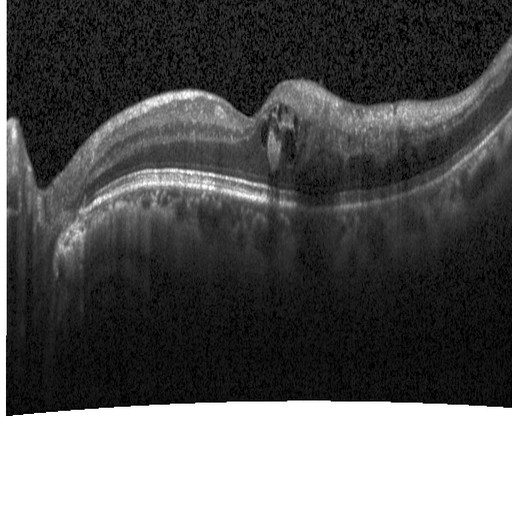

Optical coherence tomography scan
The scan shows DME.